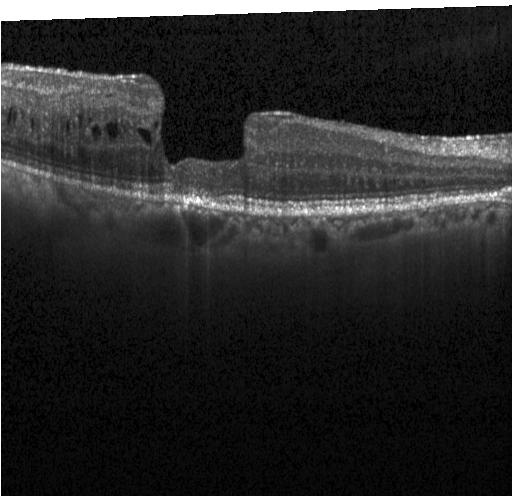

Optical coherence tomography B-scan, horizontal scan through the fovea, acquired on a Heidelberg Spectralis, SD-OCT
Macular OCT: DME.